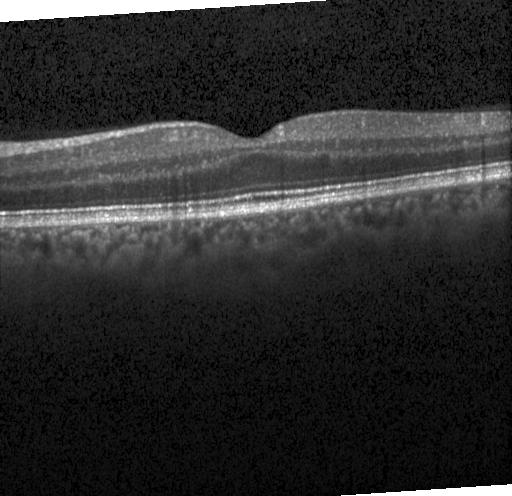

Optical coherence tomography scan · spectral-domain OCT
Dx: no evidence of CNV, DME, or drusen.